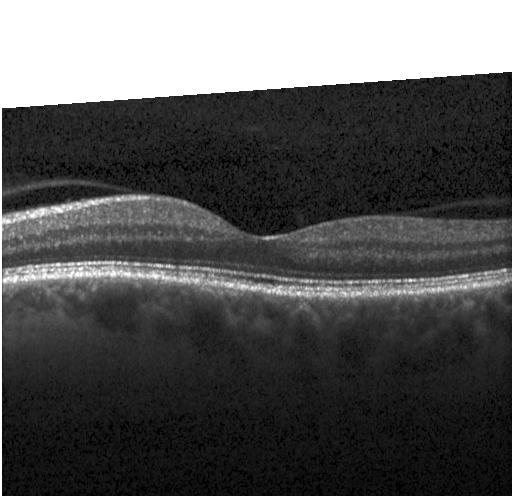

Centered on the fovea; spectral-domain OCT; acquired on a Heidelberg Spectralis; OCT B-scan. Dx: neither choroidal neovascularization, diabetic macular edema, nor drusen.